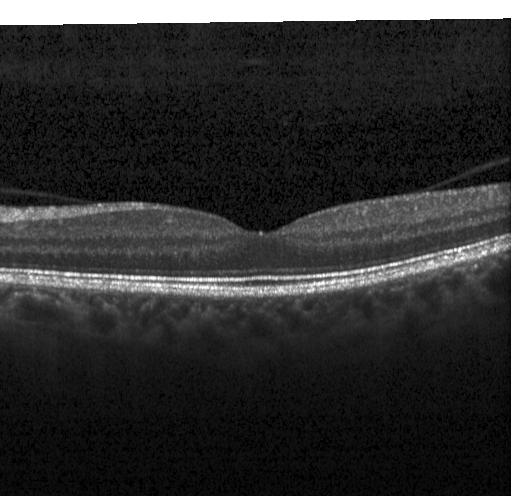 Diagnosis: no CNV, DME, or drusen.